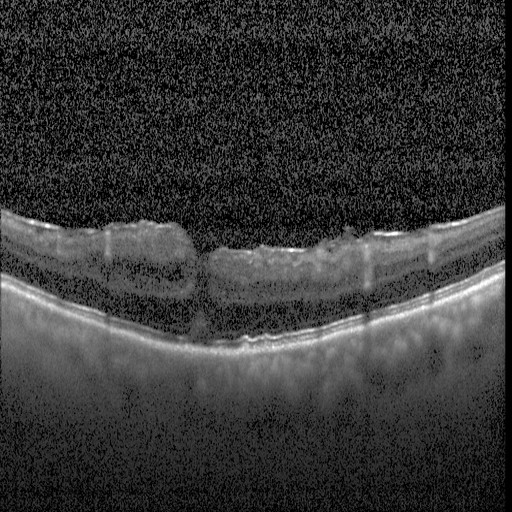

Acquired on a Heidelberg Spectralis, centered on the fovea, spectral-domain OCT, optical coherence tomography B-scan — Impression: diabetic macular edema (DME).